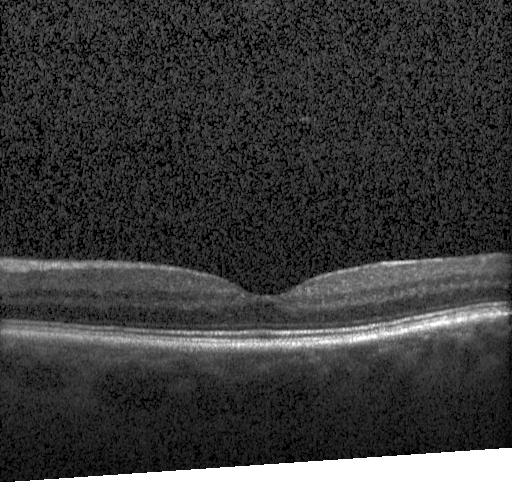
Spectral-domain OCT; macular scan; optical coherence tomography B-scan — OCT finding: no CNV, no DME, and no drusen.